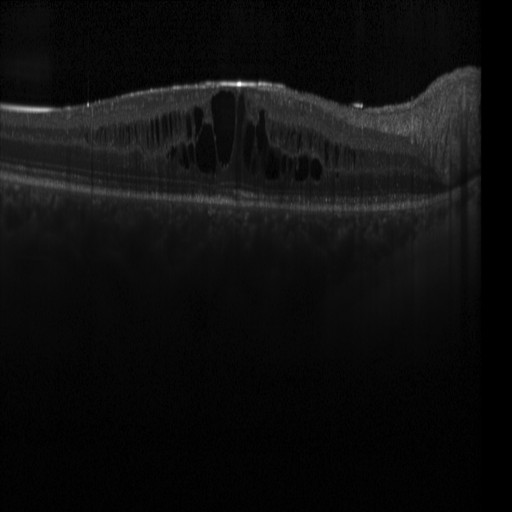
Spectral-domain OCT; macular scan; OCT B-scan; acquired on a Heidelberg Spectralis.
Diagnosis: diabetic macular edema (DME).